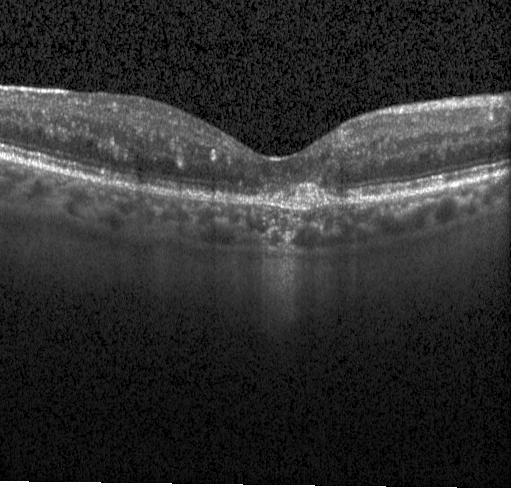
Finding: choroidal neovascularization (CNV).